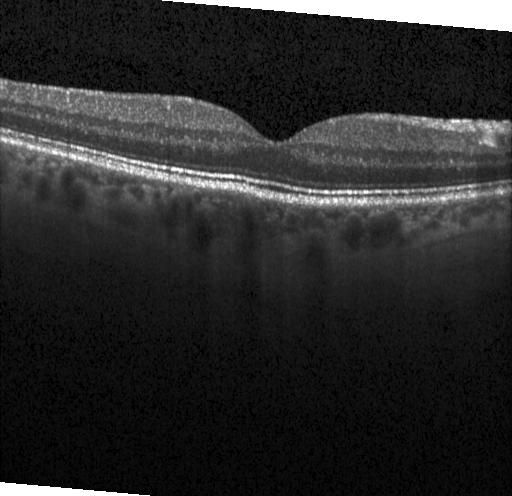

Optical coherence tomography scan. Impression: no choroidal neovascularization, diabetic macular edema, or drusen.